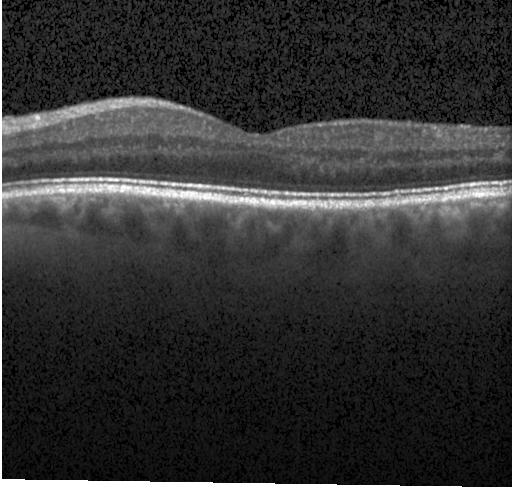
Diagnosis: no evidence of choroidal neovascularization, diabetic macular edema, or drusen.